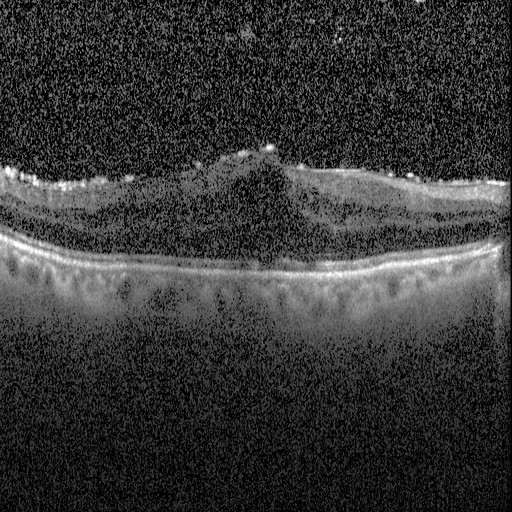

Diagnosis: diabetic macular edema (DME).